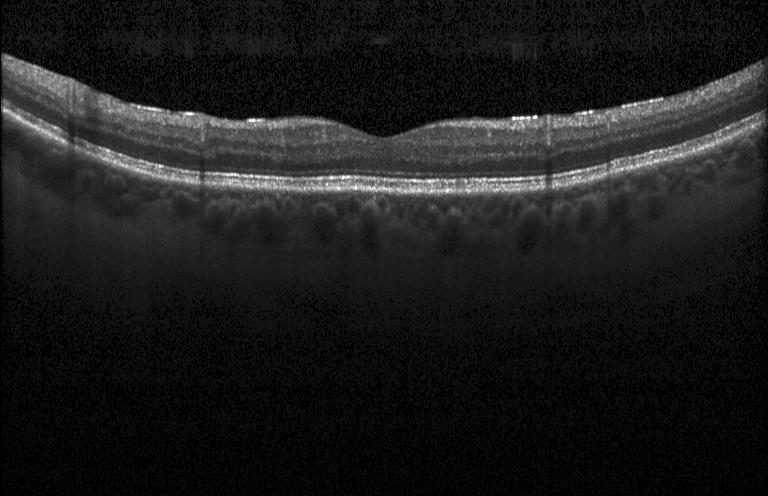 Impression: neither choroidal neovascularization, diabetic macular edema, nor drusen.